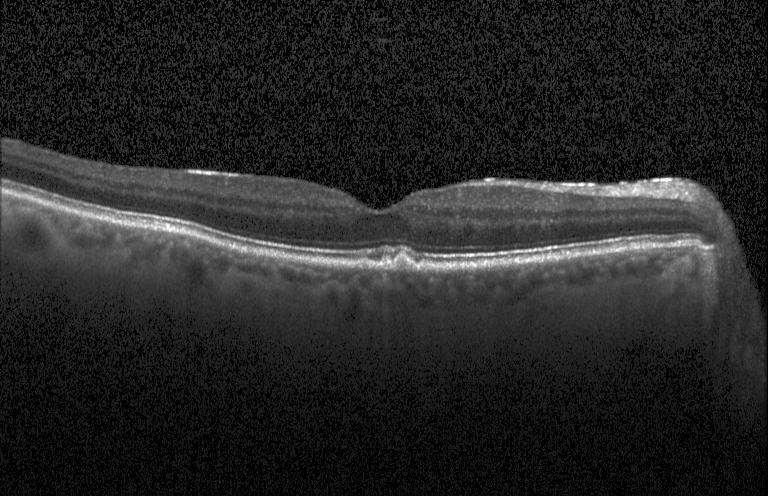 Optical coherence tomography B-scan. Finding: multiple drusen.